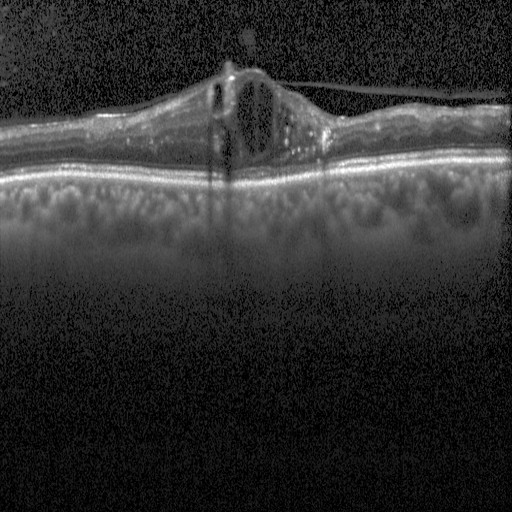
Heidelberg Spectralis OCT system; OCT B-scan.
This B-scan demonstrates DME.